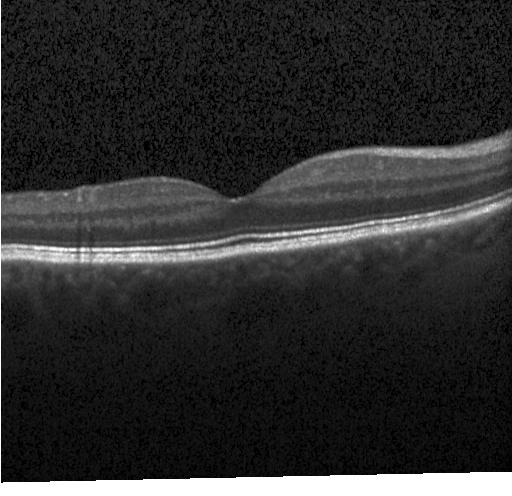
Fovea-centered, instrument: Heidelberg Spectralis, retinal OCT B-scan, spectral-domain OCT — The scan shows neither choroidal neovascularization, diabetic macular edema, nor drusen.